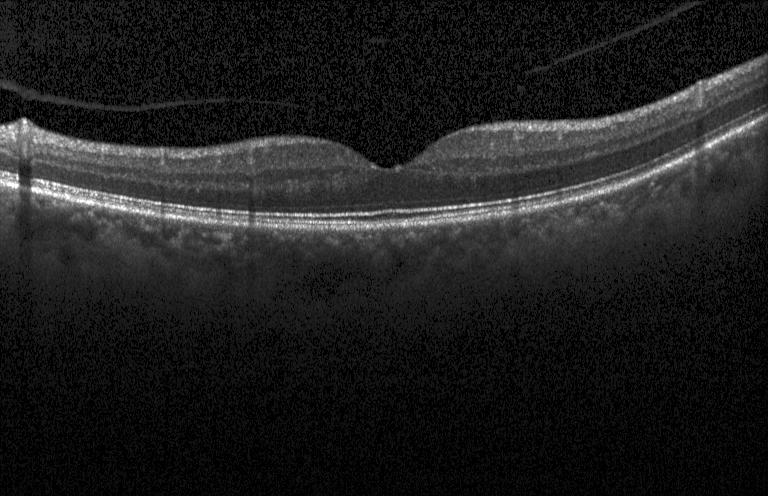 Macular OCT: no choroidal neovascularization, diabetic macular edema, or drusen.